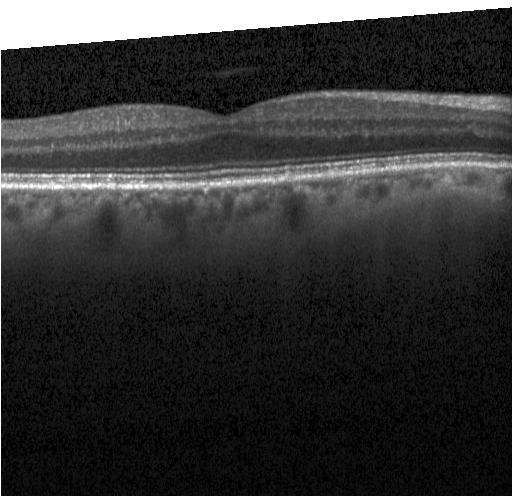 No choroidal neovascularization, no diabetic macular edema, and no drusen.